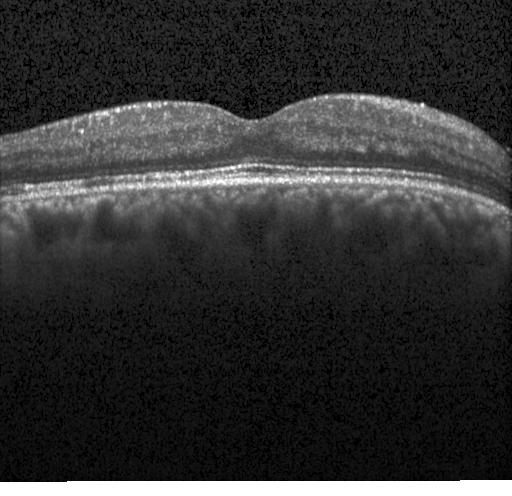
Heidelberg Spectralis OCT system; SD-OCT; optical coherence tomography B-scan; macular scan — Macular OCT: neither choroidal neovascularization, diabetic macular edema, nor drusen.